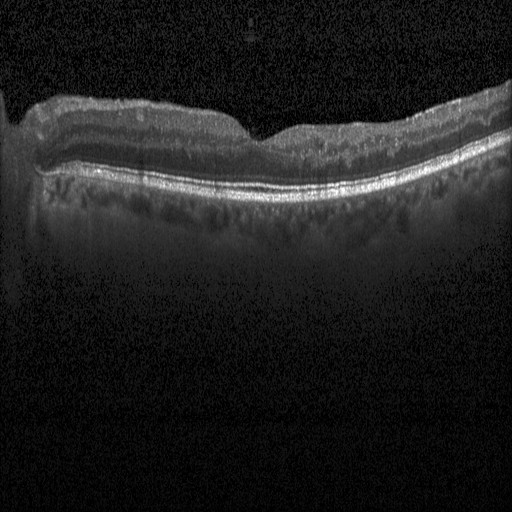 Retinal OCT cross-section. Diagnosis: DME.